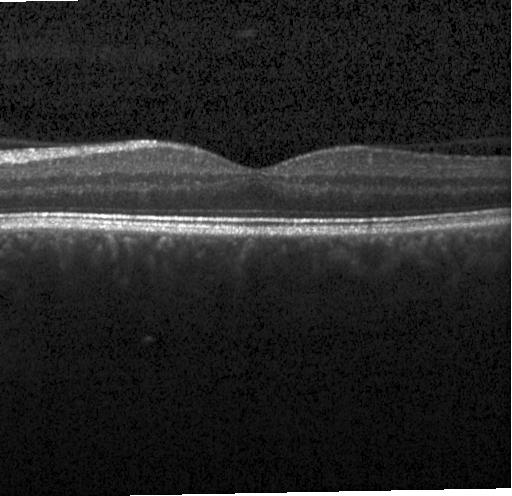 Retinal OCT cross-section. The scan shows no evidence of choroidal neovascularization, diabetic macular edema, or drusen.